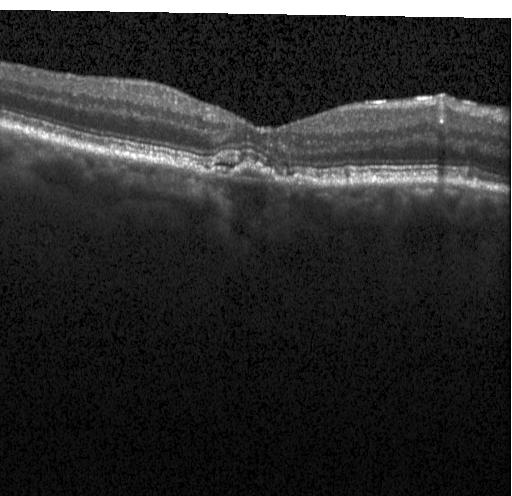
Spectral-domain OCT B-scan: a choroidal neovascular membrane.